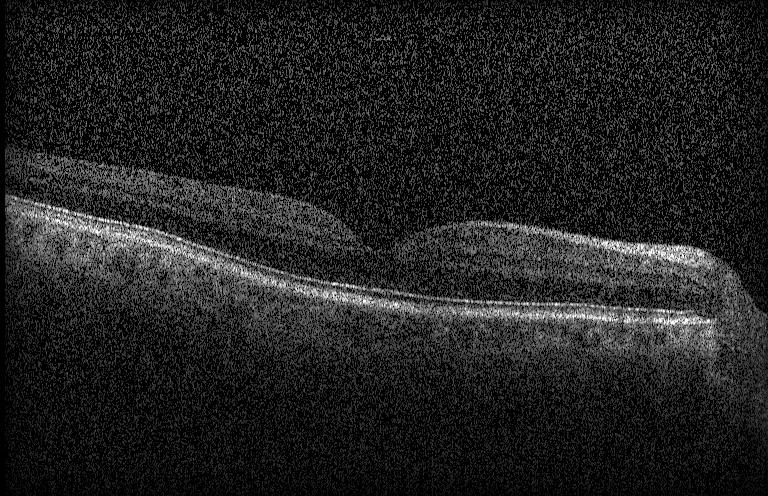
Retinal OCT cross-section showing neither choroidal neovascularization, diabetic macular edema, nor drusen.